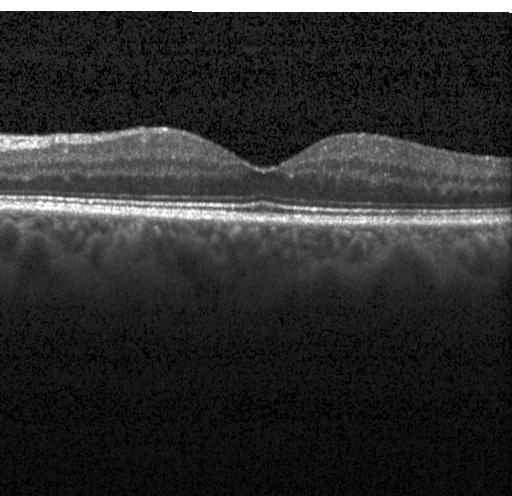
Centered on the fovea. Acquired on a Heidelberg Spectralis. Spectral-domain optical coherence tomography. Retinal OCT cross-section.
Finding: no choroidal neovascularization, no diabetic macular edema, and no drusen.